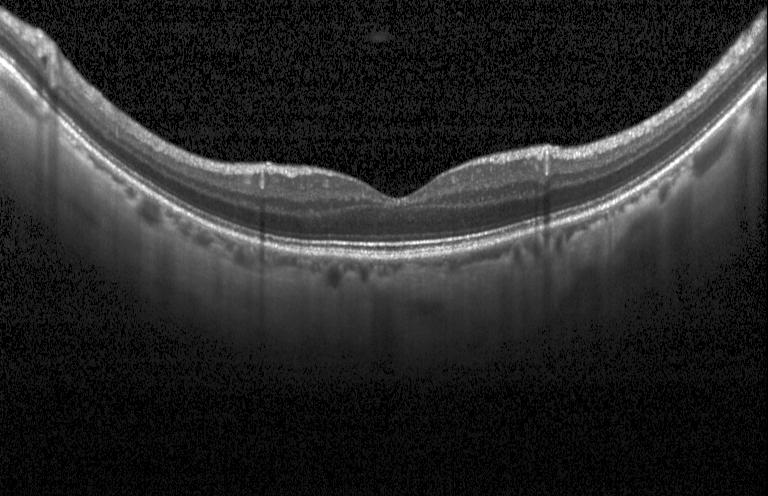

Diagnosis: no evidence of choroidal neovascularization, diabetic macular edema, or drusen.